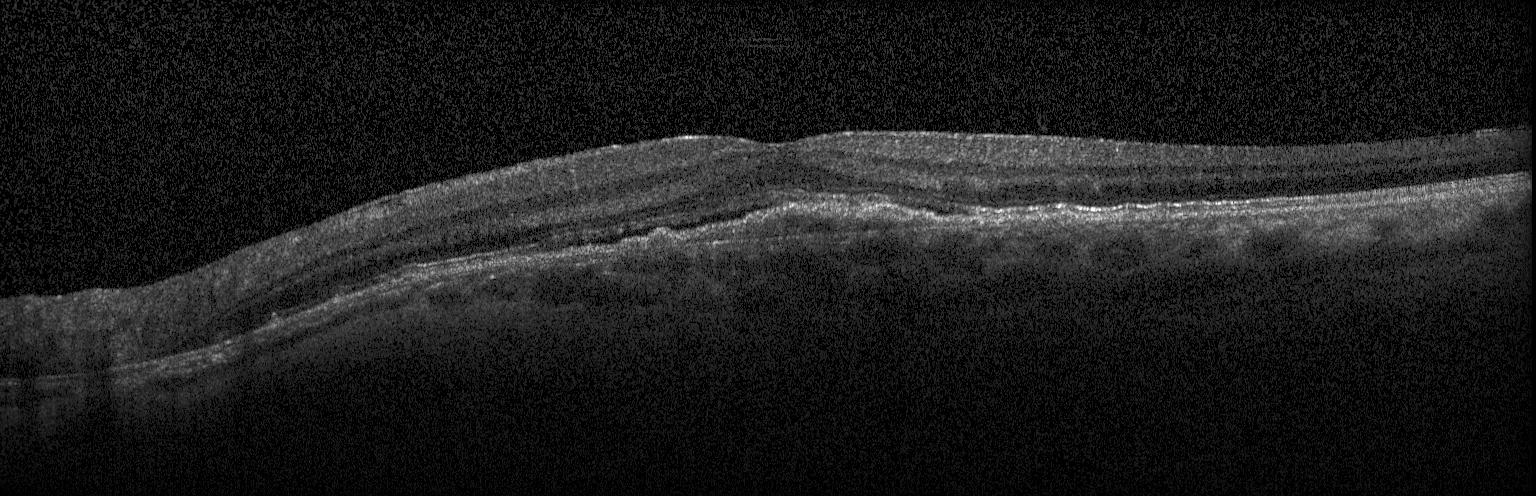 The scan shows choroidal neovascularization.